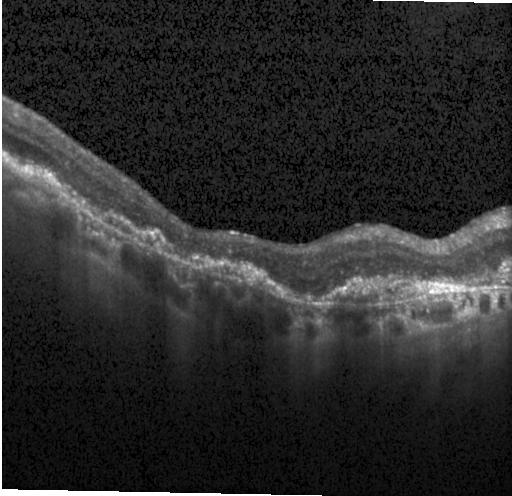
Spectral-domain optical coherence tomography, OCT B-scan, Heidelberg Spectralis.
Impression: a choroidal neovascular membrane.